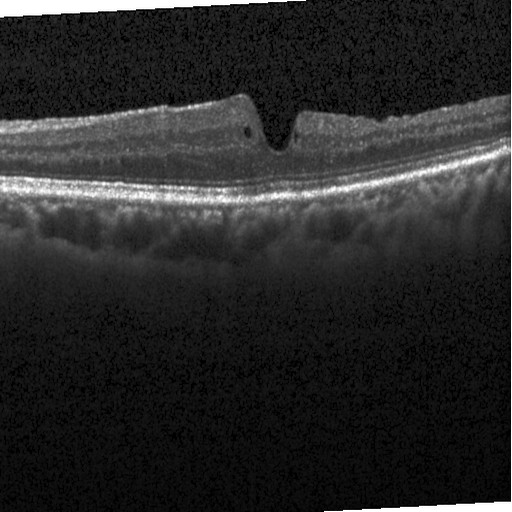
Retinal OCT cross-section. The scan shows DME.